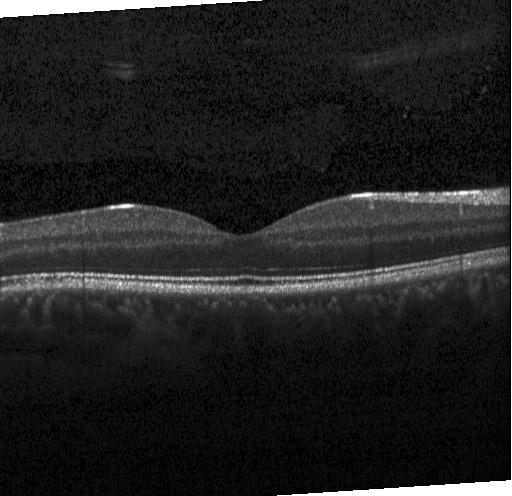
Centered on the fovea · Heidelberg Spectralis · OCT line scan · SD-OCT.
OCT finding: neither CNV, DME, nor drusen.